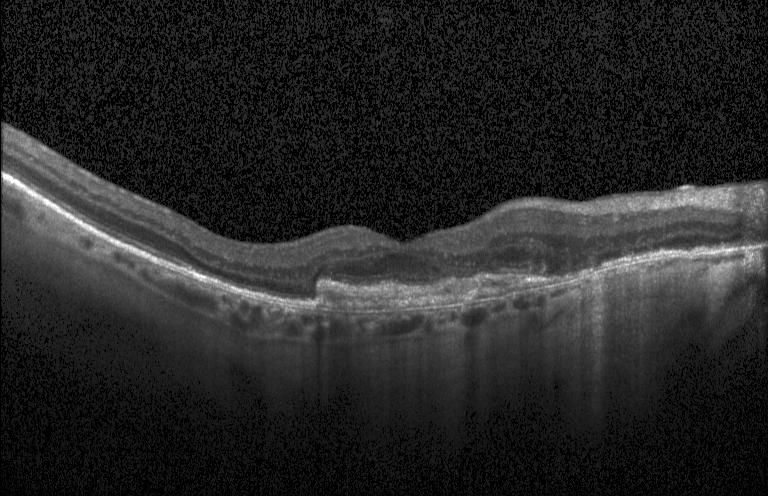
Fovea-centered; retinal OCT B-scan — Finding: a choroidal neovascular membrane.